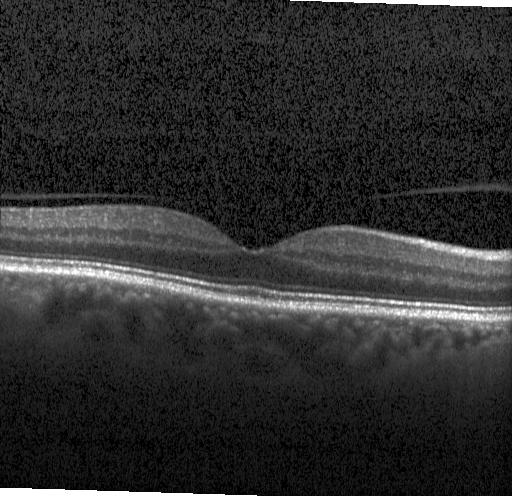
Heidelberg Spectralis OCT system, retinal OCT cross-section.
Finding: no choroidal neovascularization, no diabetic macular edema, and no drusen.